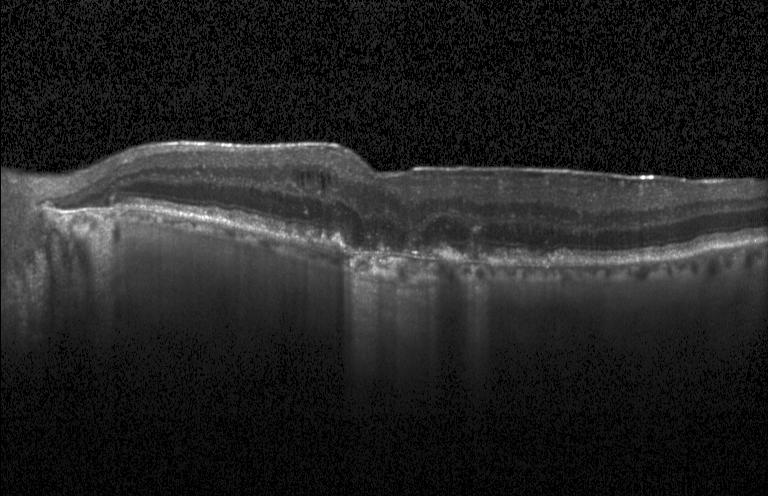

Macular OCT demonstrating CNV.